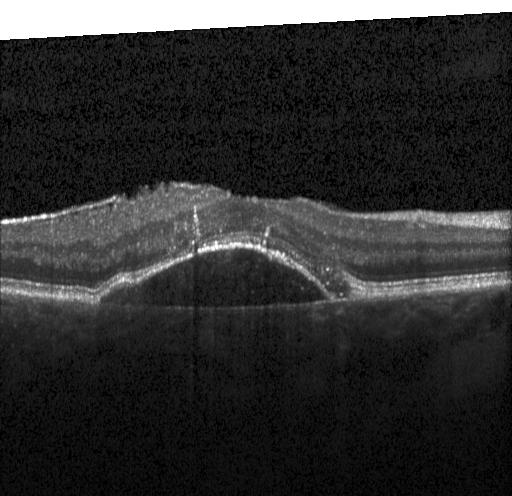 SD-OCT, through the macula, optical coherence tomography B-scan — Impression: choroidal neovascularization.